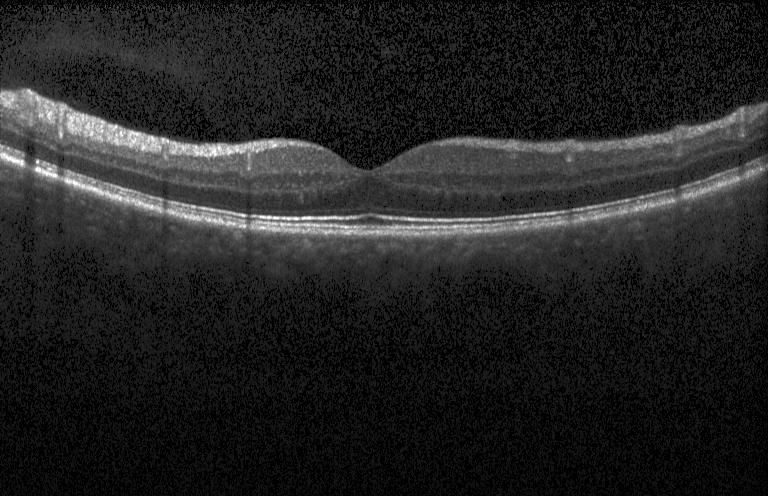

Impression: no choroidal neovascularization, no diabetic macular edema, and no drusen.